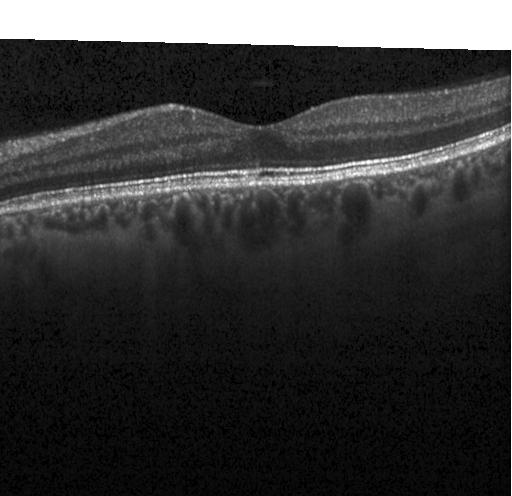 Finding: no evidence of choroidal neovascularization, diabetic macular edema, or drusen.